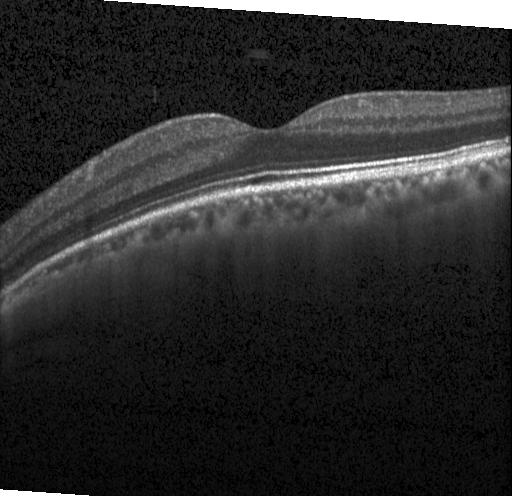
Spectral-domain OCT B-scan: neither choroidal neovascularization, diabetic macular edema, nor drusen.